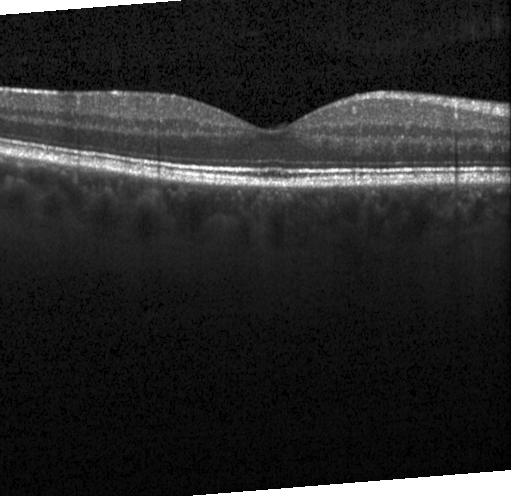
Finding: no choroidal neovascularization, no diabetic macular edema, and no drusen.